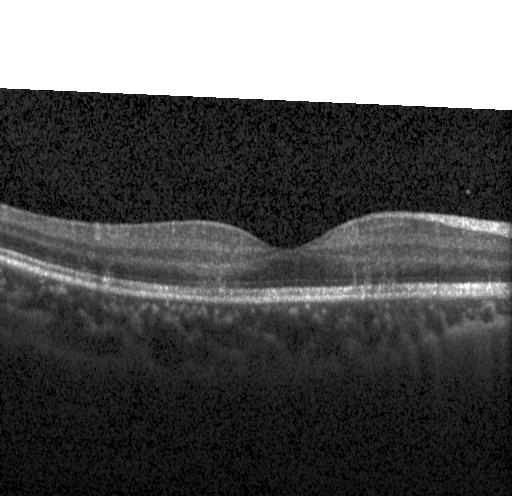 Heidelberg Spectralis · optical coherence tomography scan · macular scan · SD-OCT — Assessment: neither choroidal neovascularization, diabetic macular edema, nor drusen.